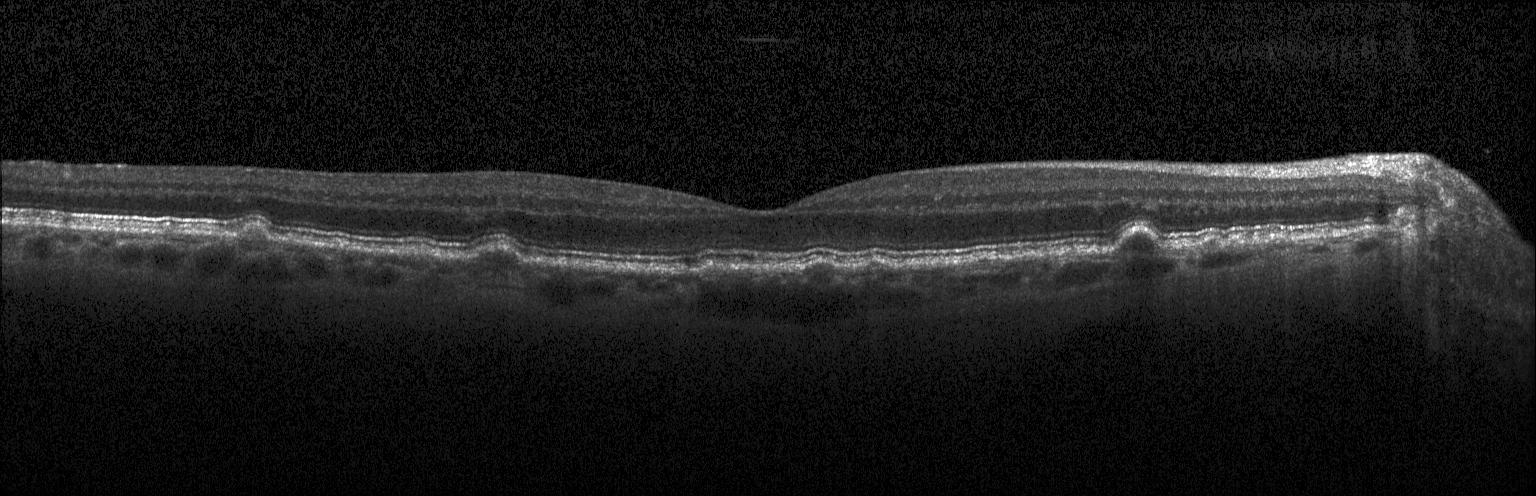

Optical coherence tomography B-scan, spectral-domain optical coherence tomography, through the macula — Diagnosis: sub-RPE drusenoid deposits.